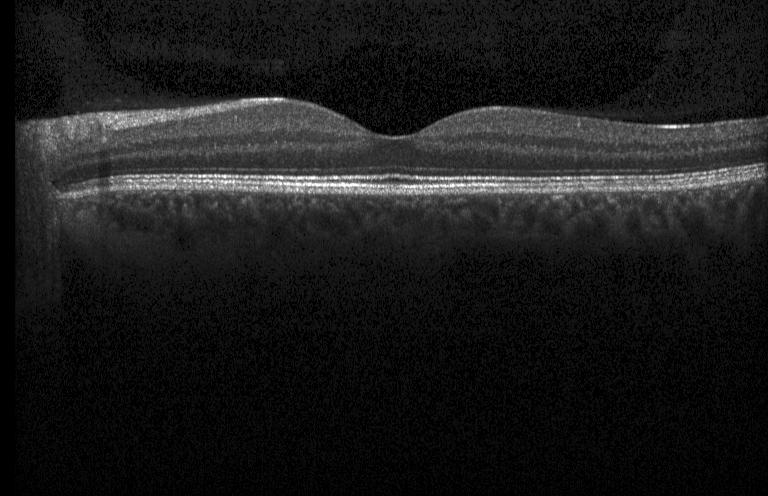 Retinal OCT cross-section showing neither CNV, DME, nor drusen.